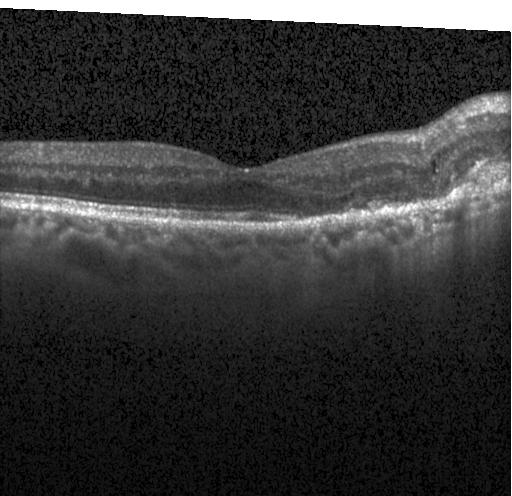

Spectral-domain OCT, acquired on a Heidelberg Spectralis, retinal OCT cross-section, horizontal scan through the fovea — Finding: a choroidal neovascular membrane.